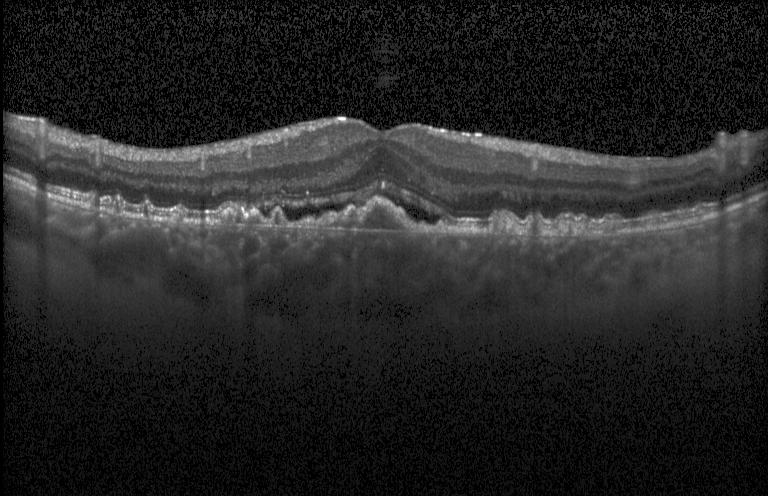
Optical coherence tomography B-scan, centered on the fovea.
Diagnosis: CNV.